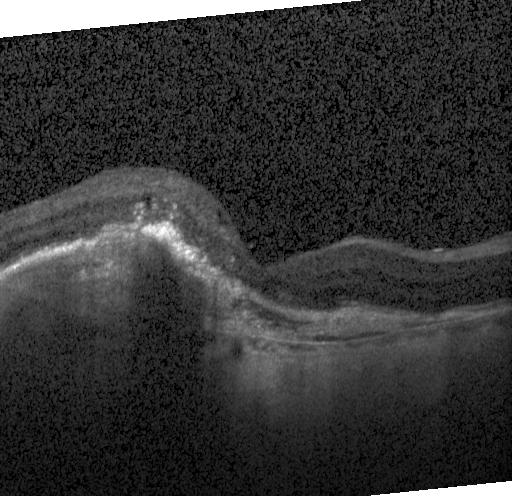 Acquired on a Heidelberg Spectralis. Optical coherence tomography B-scan. Spectral-domain OCT. Fovea-centered — Macular OCT: a choroidal neovascular membrane.